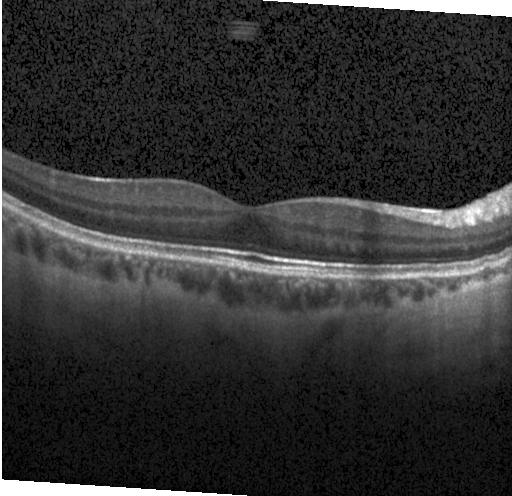

Centered on the fovea, OCT line scan — Finding: neither CNV, DME, nor drusen.